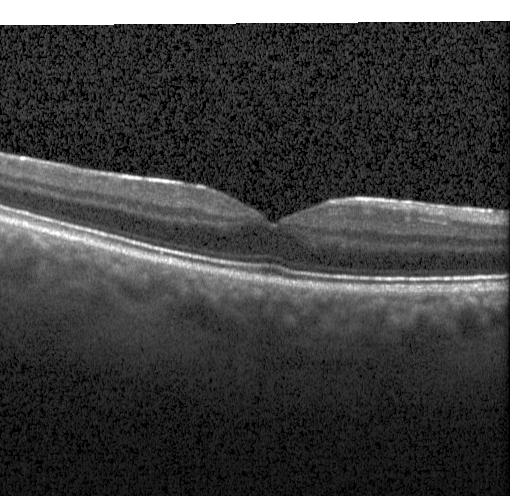
Assessment: no evidence of CNV, DME, or drusen.